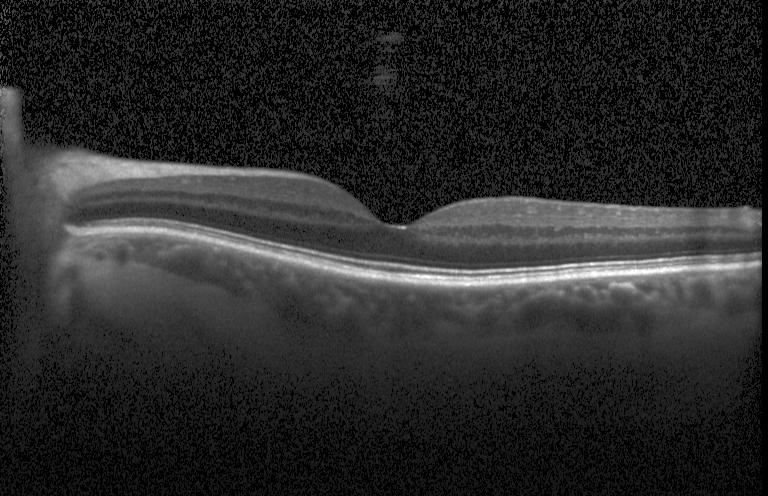 Macular OCT: no choroidal neovascularization, diabetic macular edema, or drusen.